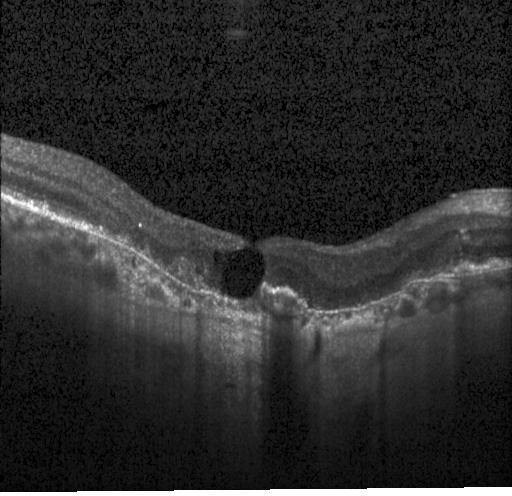

Heidelberg Spectralis · optical coherence tomography B-scan · centered on the fovea · spectral-domain optical coherence tomography.
Finding: CNV.